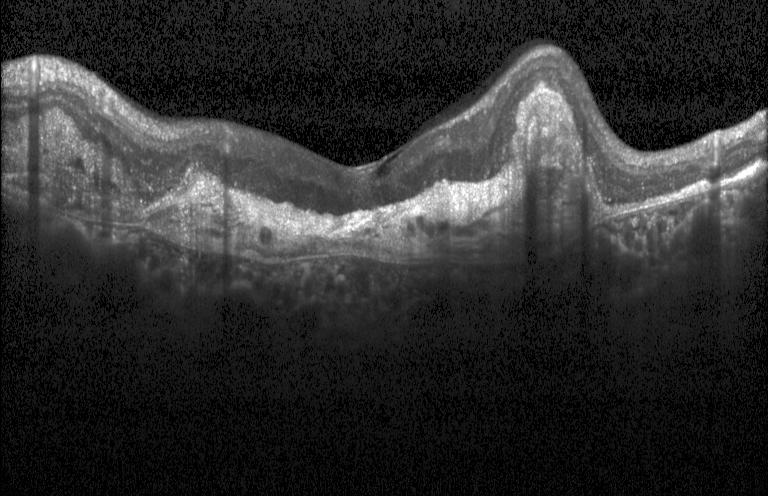 OCT finding: a choroidal neovascular membrane.